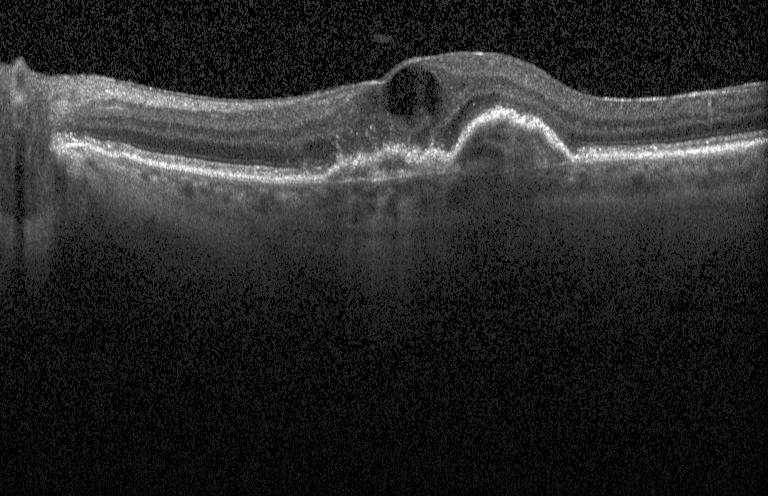
Retinal OCT B-scan, spectral-domain OCT, instrument: Heidelberg Spectralis, horizontal scan through the fovea — Diagnosis: a choroidal neovascular membrane.